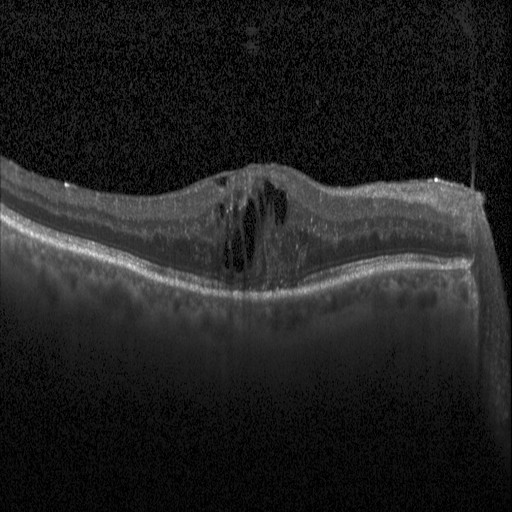 Retinal OCT B-scan; Heidelberg Spectralis OCT system; through the macula; spectral-domain optical coherence tomography. Impression: diabetic macular edema (DME).